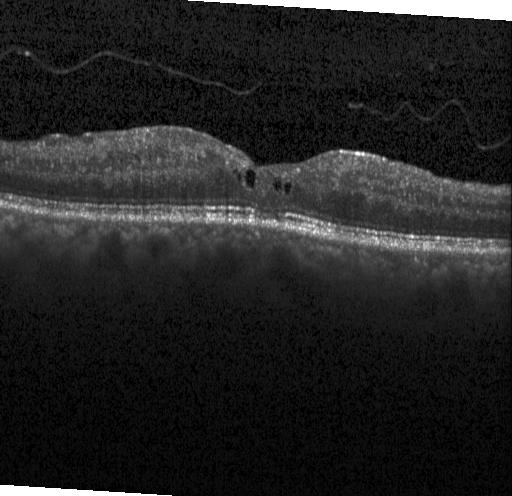 Optical coherence tomography B-scan
Impression: DME.